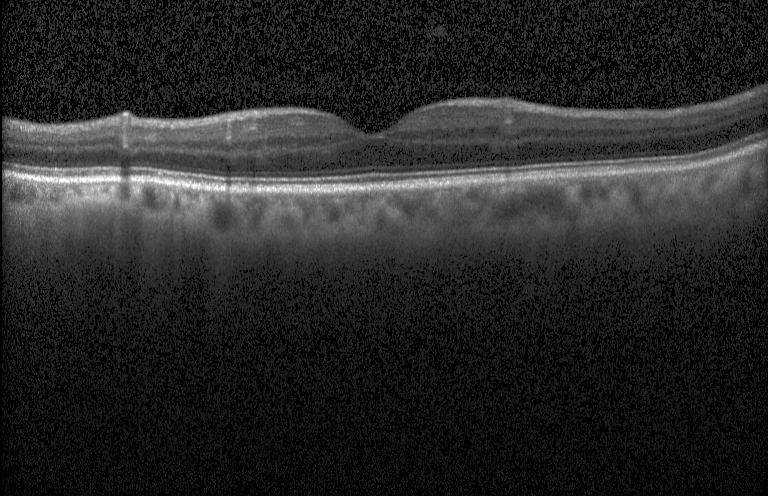
Retinal OCT cross-section showing no CNV, DME, or drusen.